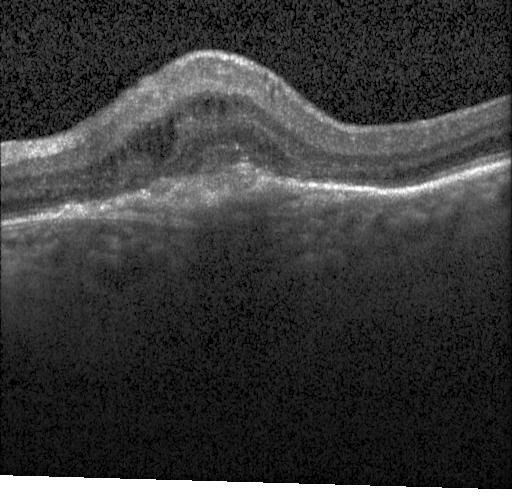

A choroidal neovascular membrane.